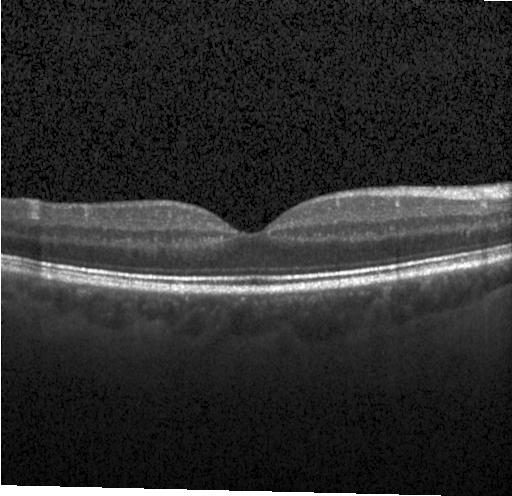 Optical coherence tomography B-scan, spectral-domain OCT — Impression: no choroidal neovascularization, no diabetic macular edema, and no drusen.